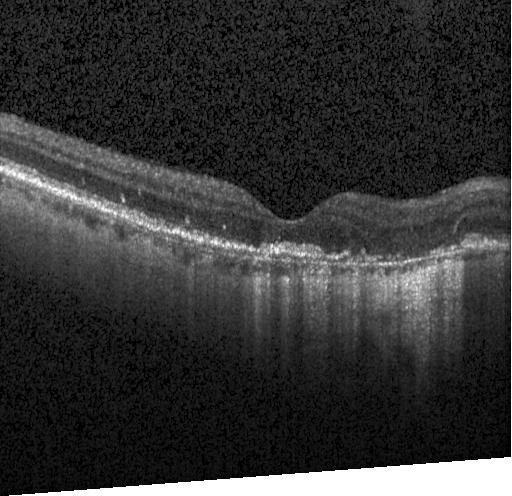
OCT B-scan showing a choroidal neovascular membrane.